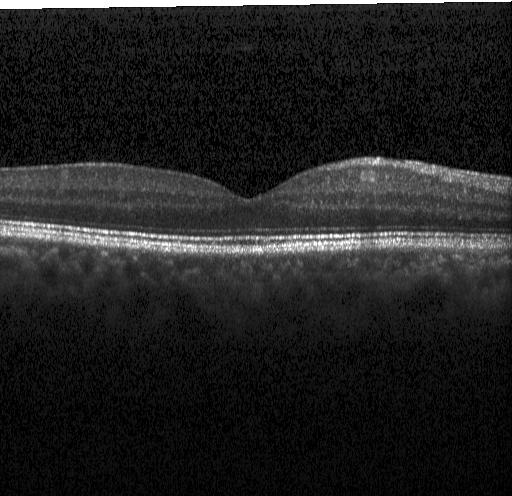

Optical coherence tomography B-scan. Instrument: Heidelberg Spectralis. Horizontal scan through the fovea
Diagnosis: no choroidal neovascularization, diabetic macular edema, or drusen.